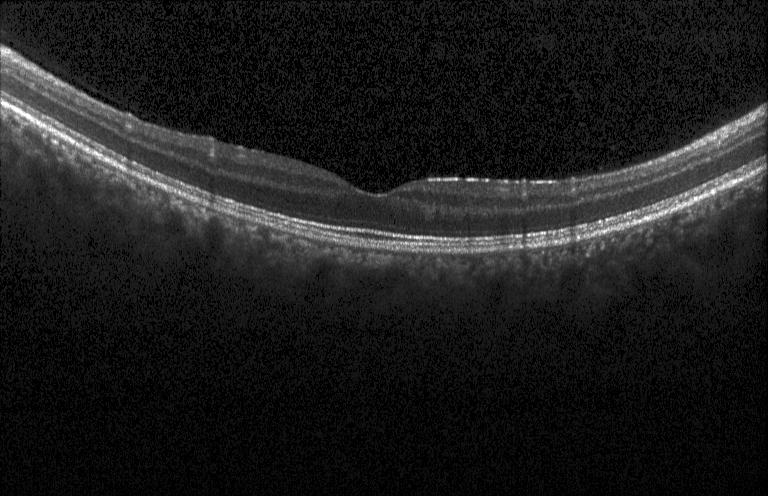
Macular scan, acquired on a Heidelberg Spectralis, spectral-domain optical coherence tomography, optical coherence tomography B-scan. Impression: no CNV, no DME, and no drusen.